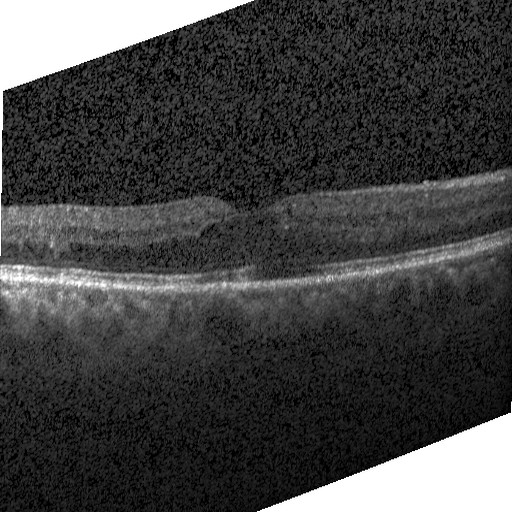

Retinal OCT cross-section. Diagnosis: diabetic macular edema (DME).